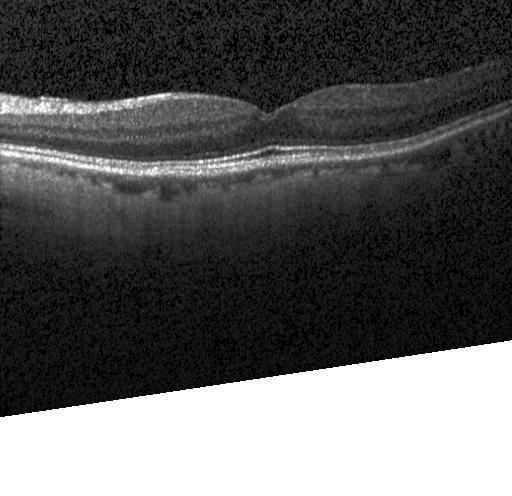

This B-scan demonstrates no choroidal neovascularization, no diabetic macular edema, and no drusen.